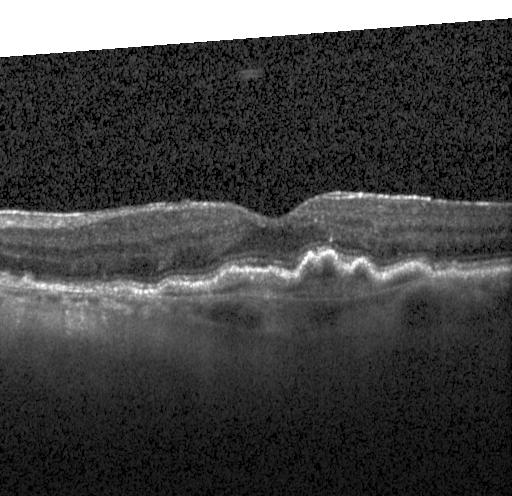

Impression: a choroidal neovascular membrane.